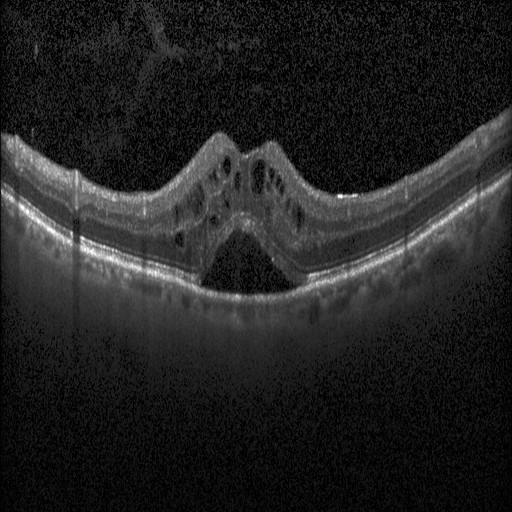
Retinal OCT cross-section; Heidelberg Spectralis OCT system
Finding: diabetic macular edema (DME).